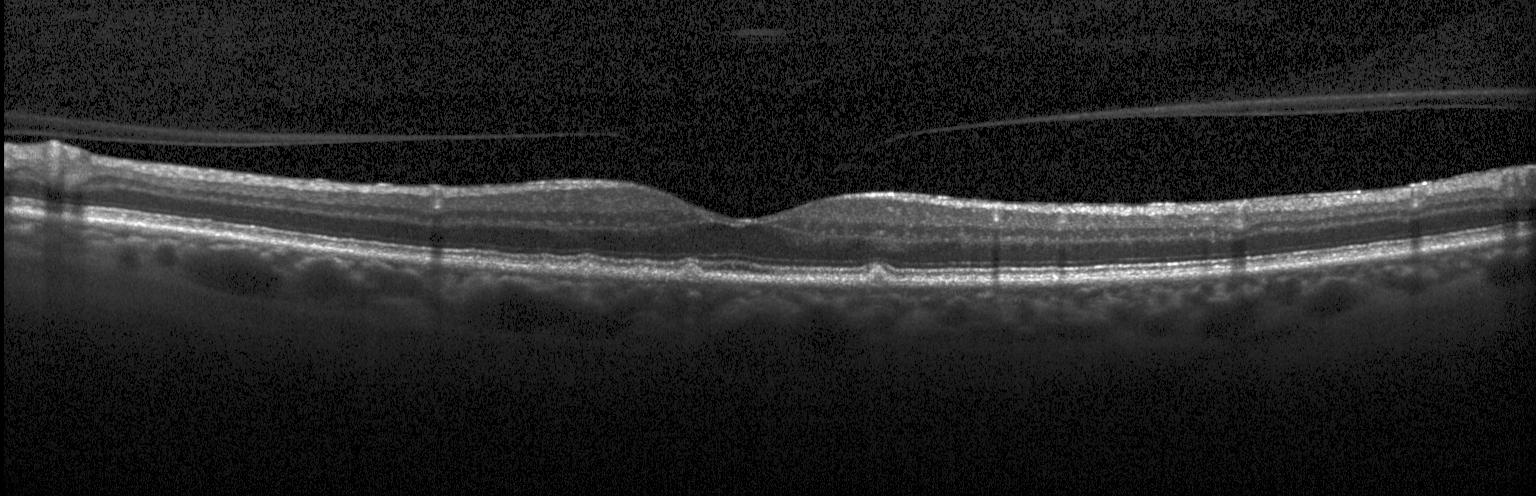
Heidelberg Spectralis · OCT B-scan.
Finding: drusen.